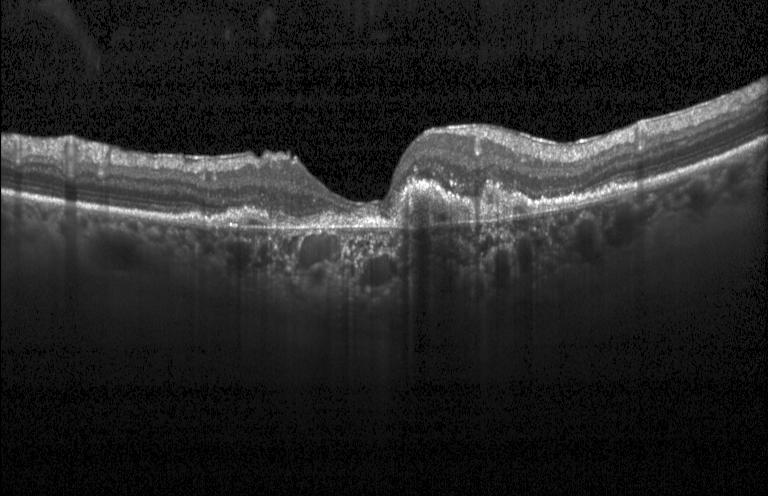

OCT line scan · SD-OCT · acquired on a Heidelberg Spectralis. Assessment: choroidal neovascularization (CNV).